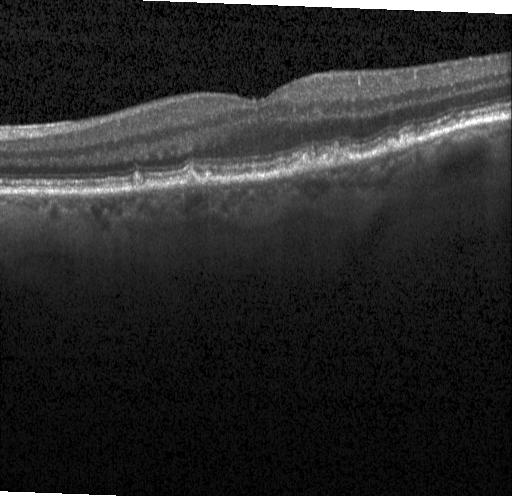
Retinal OCT B-scan. Impression: drusen.